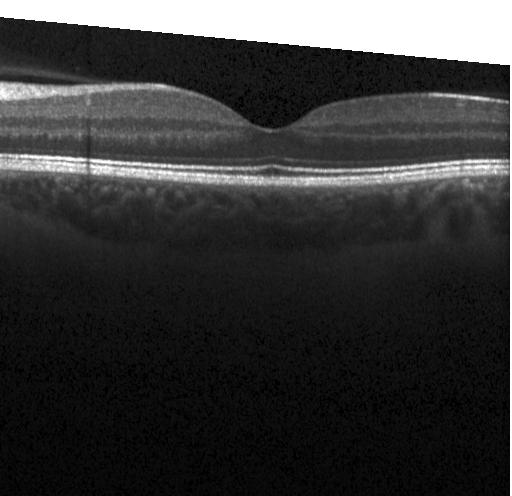
OCT line scan.
Macular OCT: no evidence of CNV, DME, or drusen.